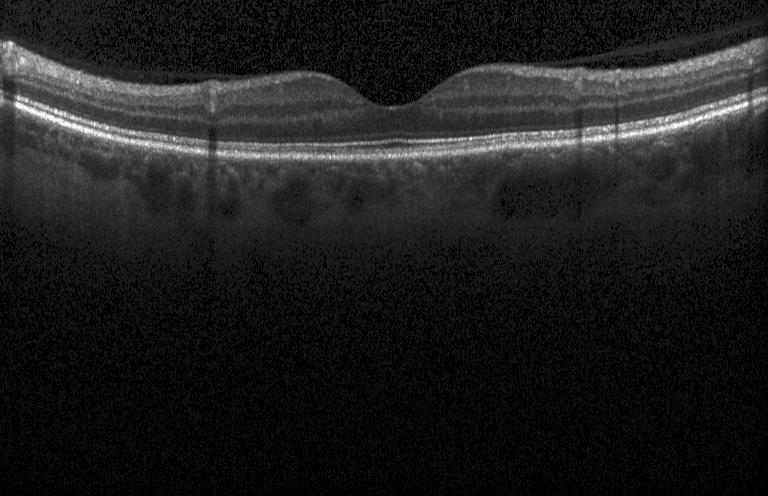 OCT finding: no choroidal neovascularization, diabetic macular edema, or drusen.